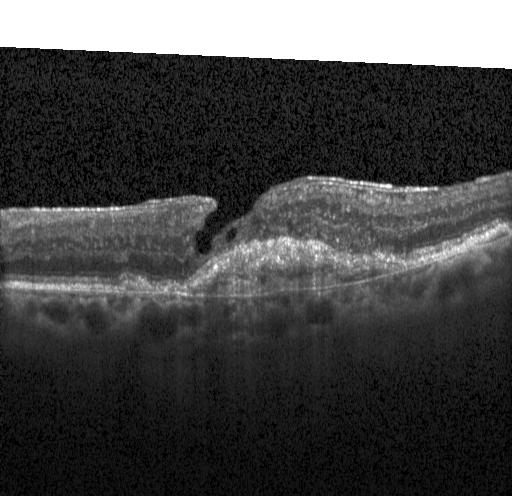

Finding: choroidal neovascularization (CNV).